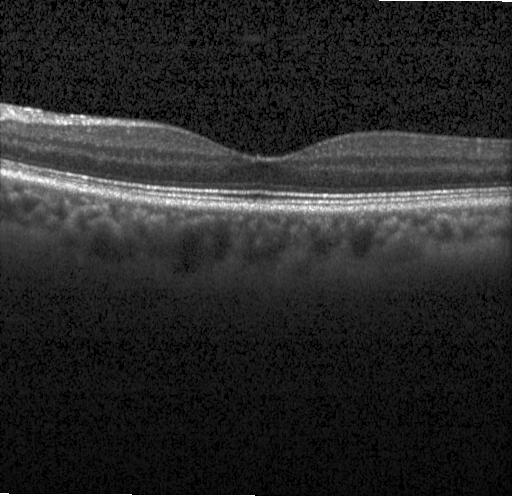
Retinal OCT cross-section — Dx: no evidence of choroidal neovascularization, diabetic macular edema, or drusen.